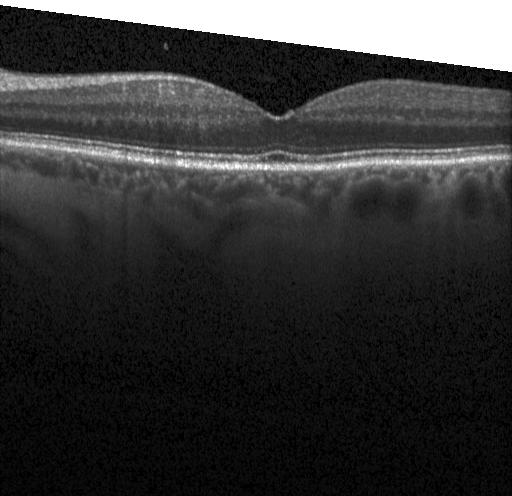
Diagnosis: neither CNV, DME, nor drusen.